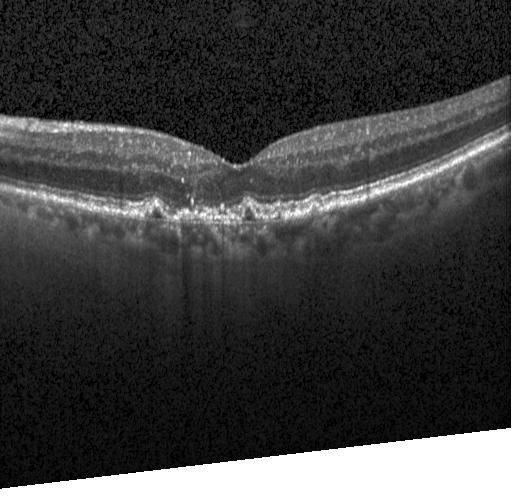
Macular OCT demonstrating choroidal neovascularization.